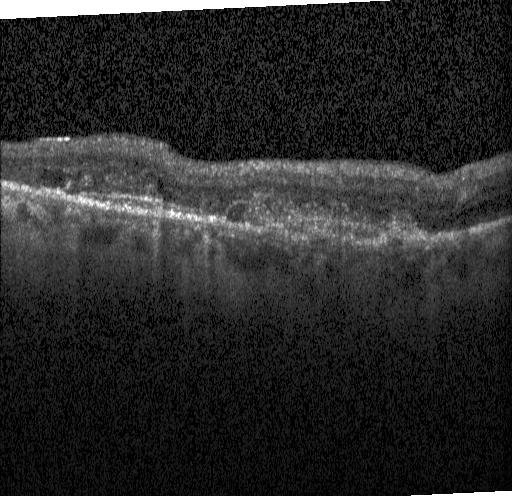 OCT B-scan. The scan shows CNV.